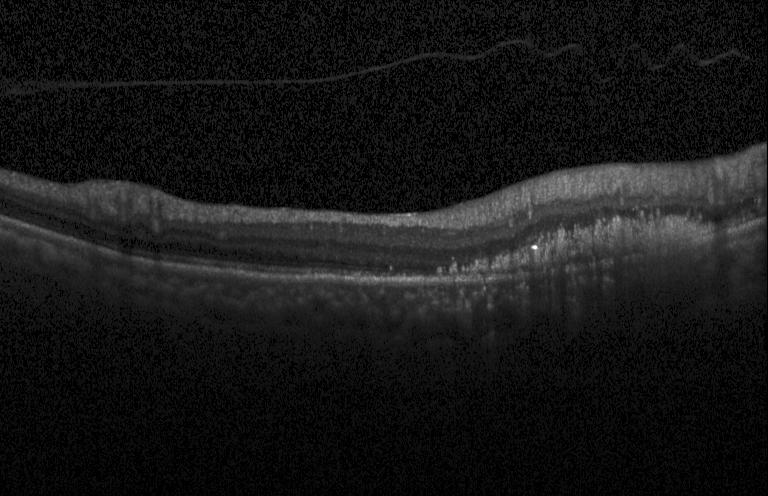 Centered on the fovea. Spectral-domain OCT. Optical coherence tomography scan. Diagnosis: choroidal neovascularization.